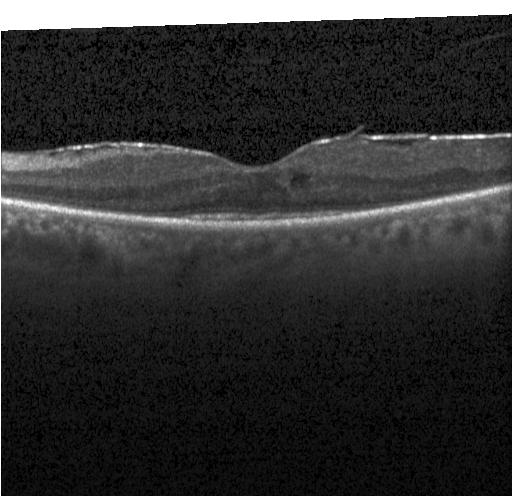

OCT B-scan. SD-OCT
This B-scan demonstrates diabetic macular edema.